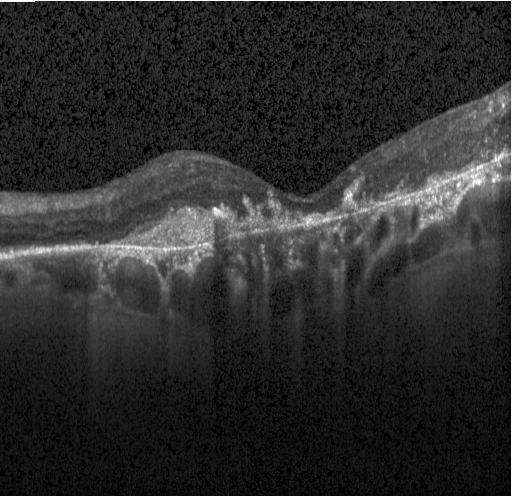

Diagnosis: choroidal neovascularization (CNV).